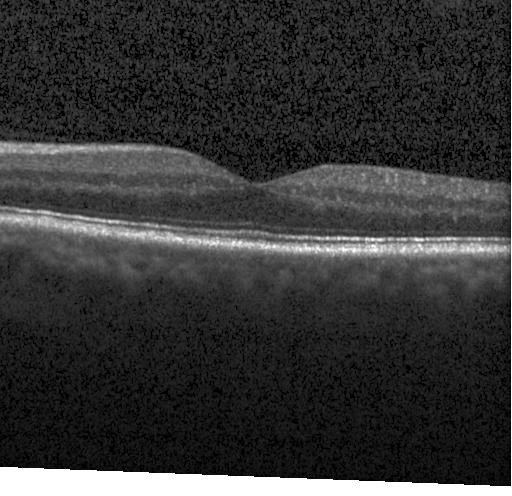
Diagnosis: no CNV, DME, or drusen.